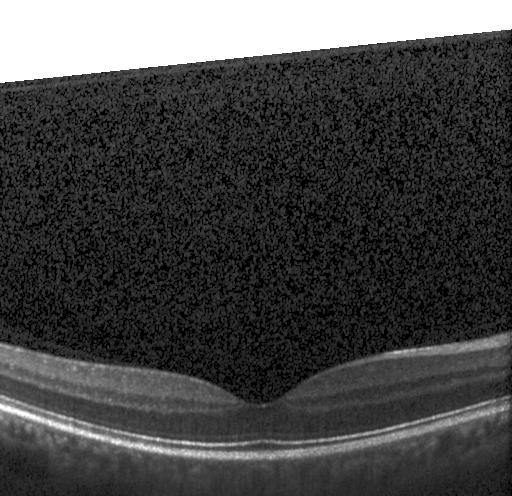

Optical coherence tomography scan. Centered on the fovea. Acquired on a Heidelberg Spectralis
Impression: no evidence of CNV, DME, or drusen.